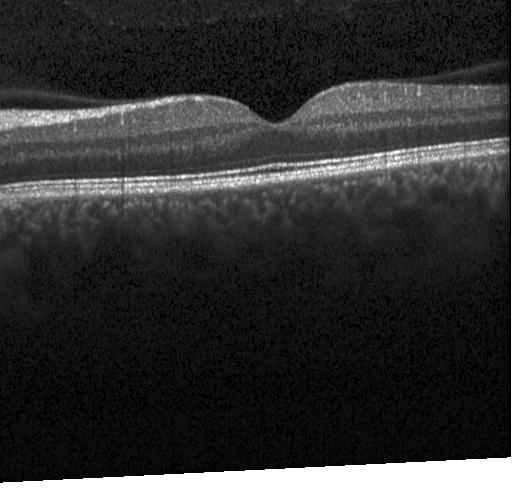

Impression: neither choroidal neovascularization, diabetic macular edema, nor drusen.